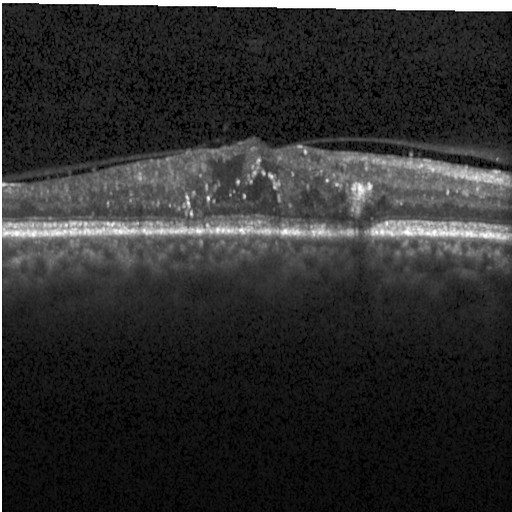 This B-scan demonstrates diabetic macular edema.